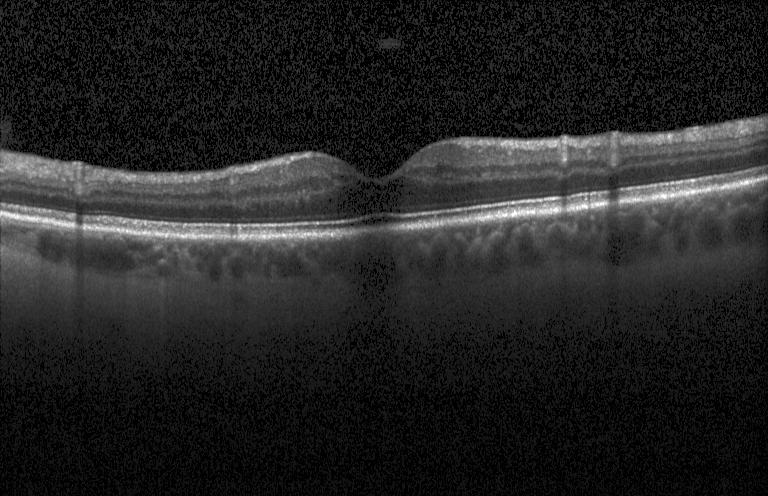

Macular OCT: no CNV, no DME, and no drusen.